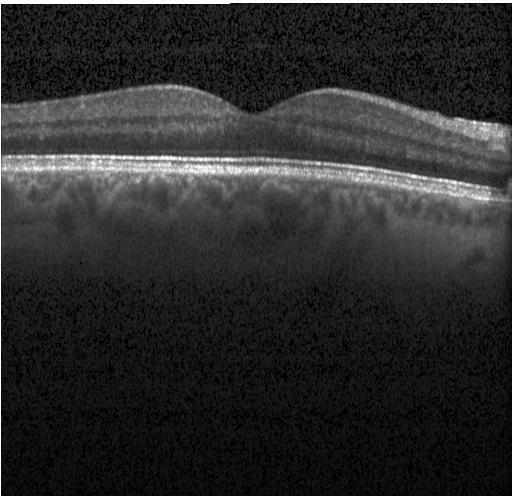

Retinal OCT B-scan. Horizontal scan through the fovea. Heidelberg Spectralis OCT system. Spectral-domain OCT
The scan shows neither choroidal neovascularization, diabetic macular edema, nor drusen.